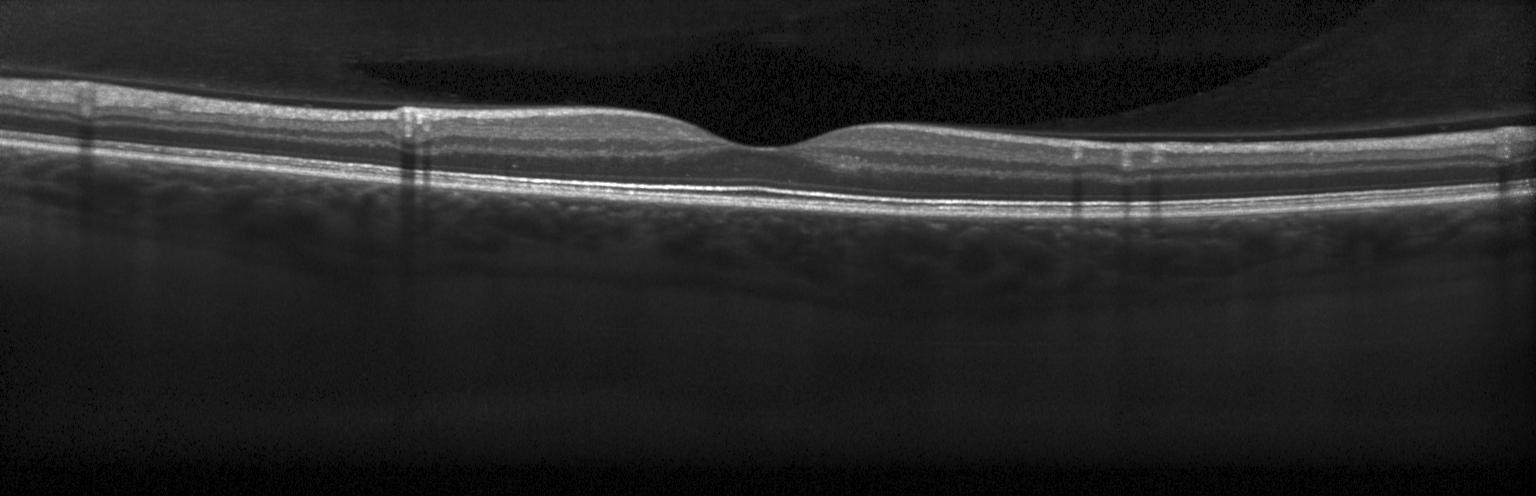
OCT line scan — OCT finding: no CNV, no DME, and no drusen.